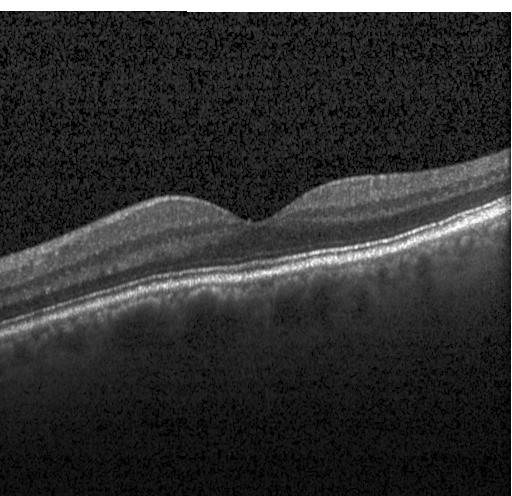 OCT B-scan showing no choroidal neovascularization, diabetic macular edema, or drusen.